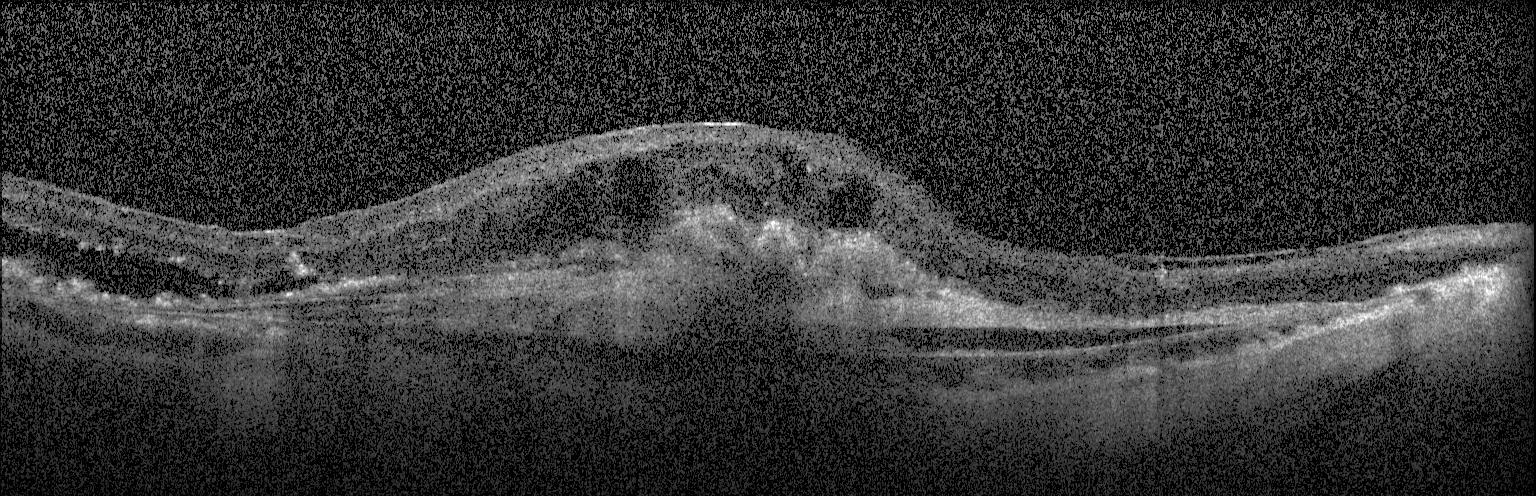
Retinal OCT B-scan, SD-OCT
Finding: a choroidal neovascular membrane.